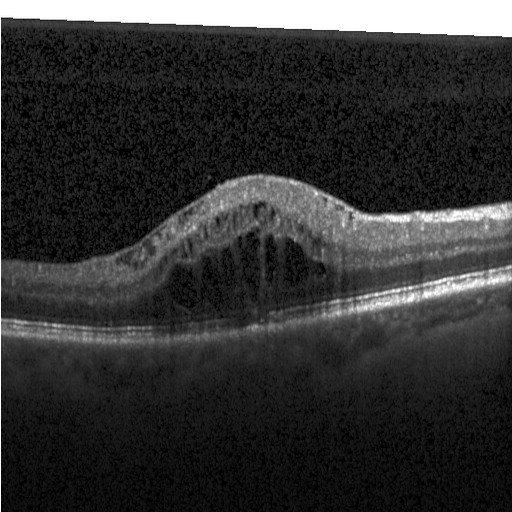 Fovea-centered; Heidelberg Spectralis; retinal OCT B-scan.
Diabetic macular edema.